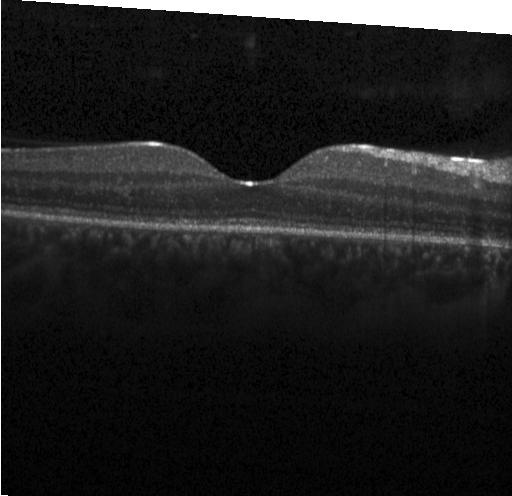

Retinal OCT B-scan. Acquired on a Heidelberg Spectralis. Fovea-centered
Diagnosis: no choroidal neovascularization, diabetic macular edema, or drusen.